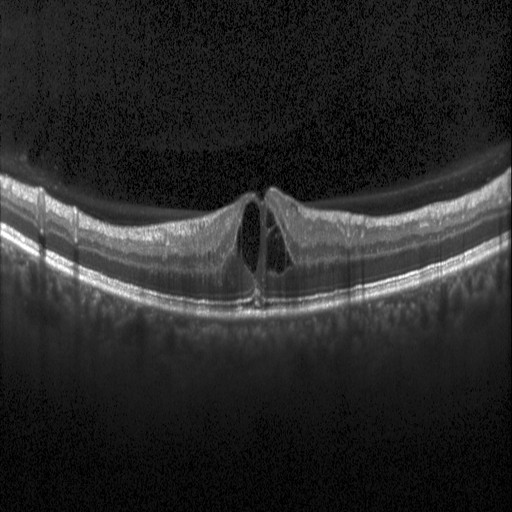

Dx: diabetic macular edema (DME).